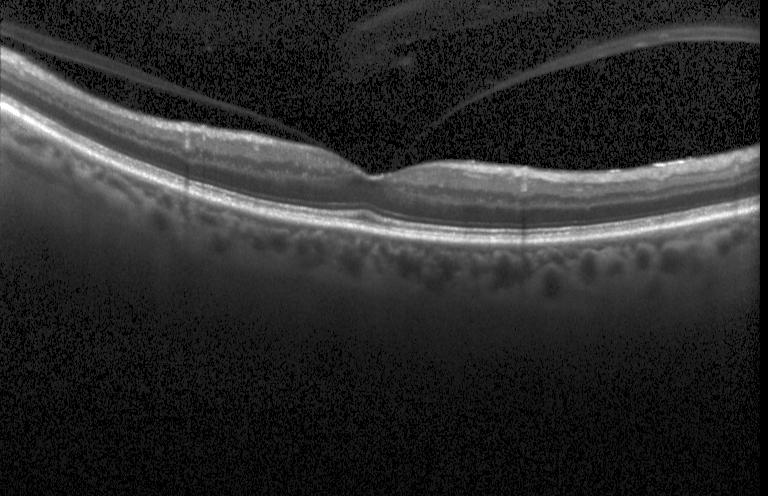
SD-OCT. Optical coherence tomography B-scan. No choroidal neovascularization, no diabetic macular edema, and no drusen.